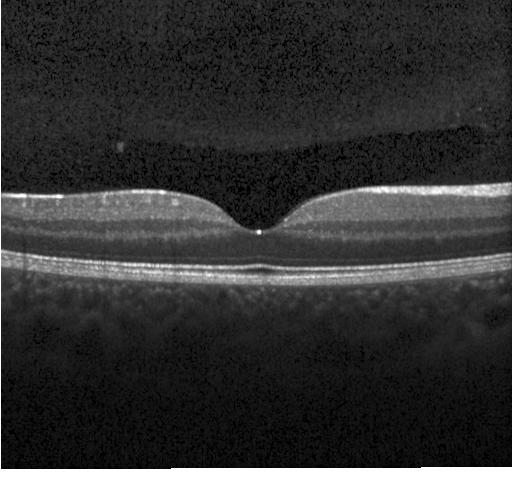

Optical coherence tomography scan. Instrument: Heidelberg Spectralis. Diagnosis: no choroidal neovascularization, no diabetic macular edema, and no drusen.